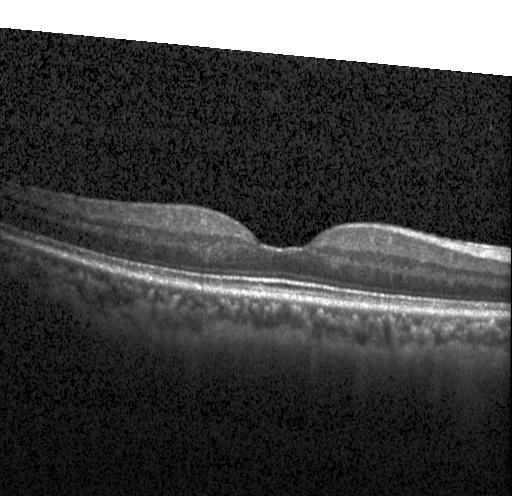 Macular scan, OCT line scan. OCT finding: no choroidal neovascularization, diabetic macular edema, or drusen.